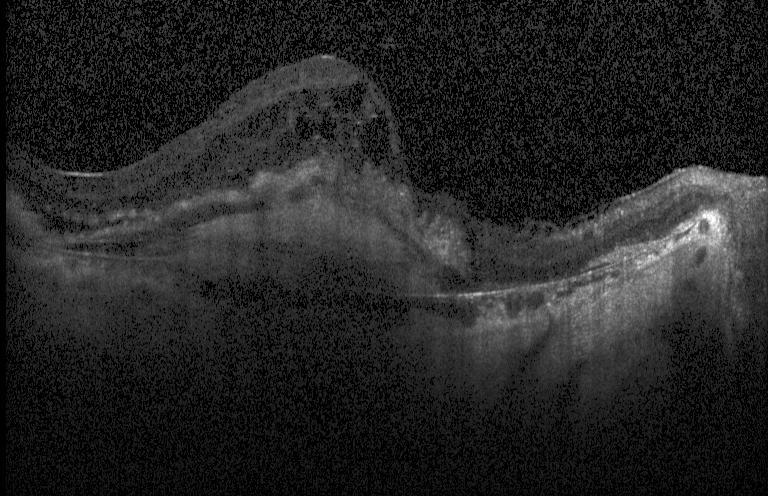 Diagnosis: a choroidal neovascular membrane.